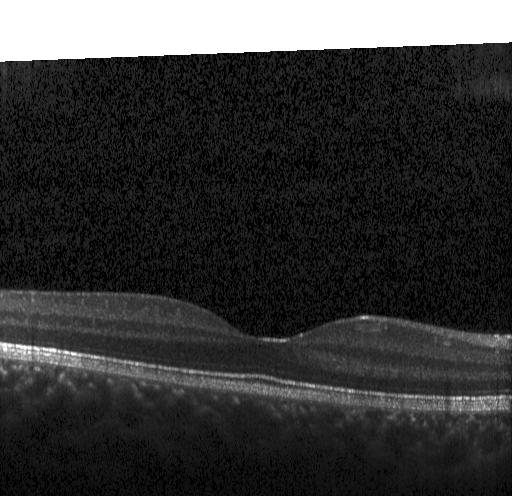

OCT B-scan showing no CNV, DME, or drusen.